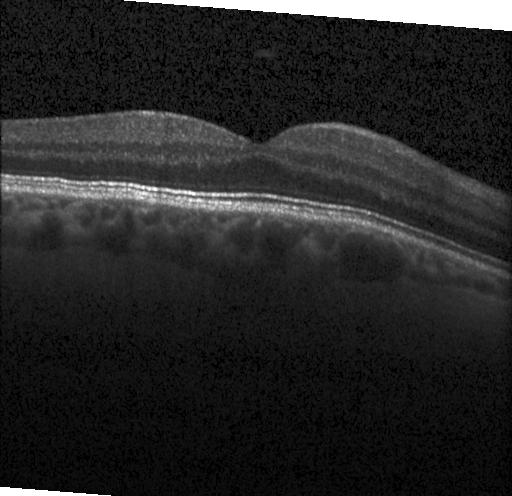
OCT line scan — No choroidal neovascularization, no diabetic macular edema, and no drusen.